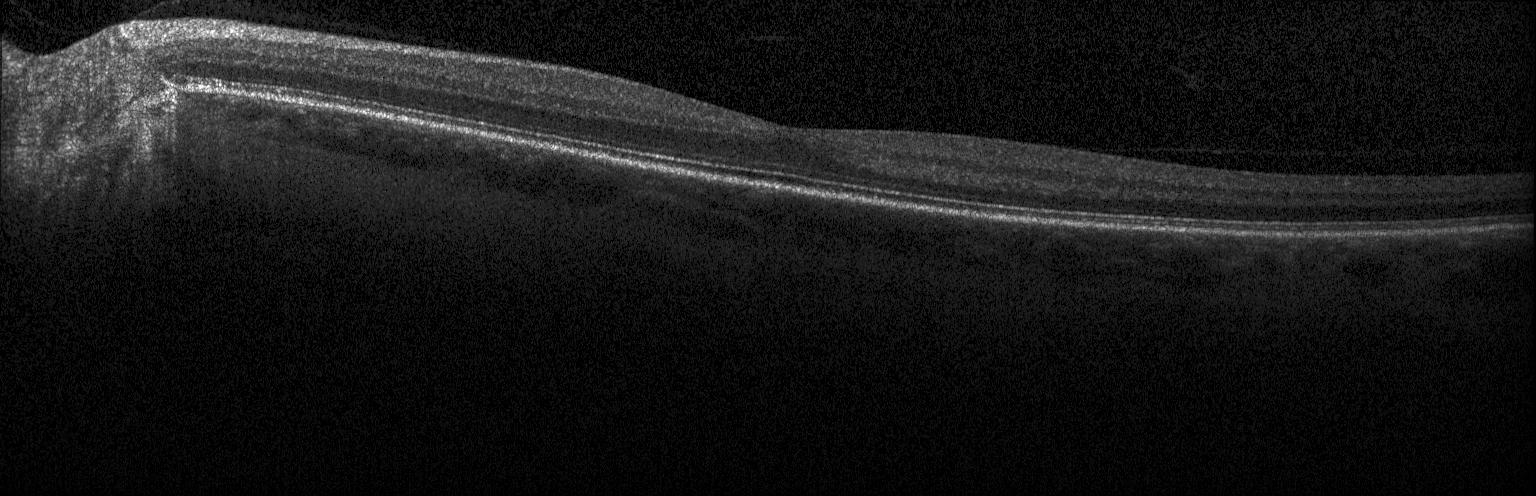

Heidelberg Spectralis OCT system; OCT B-scan; SD-OCT. Macular OCT: no evidence of choroidal neovascularization, diabetic macular edema, or drusen.